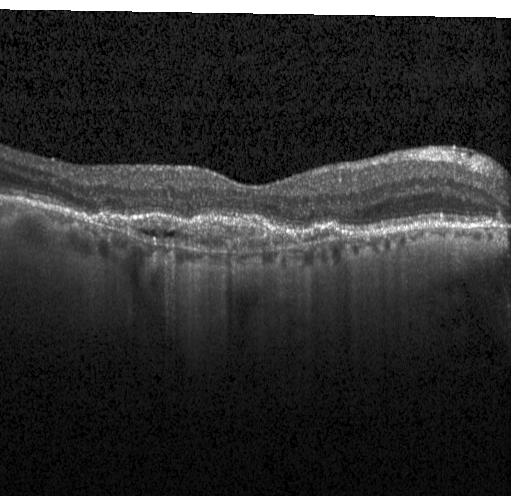 OCT B-scan. Dx: choroidal neovascularization (CNV).